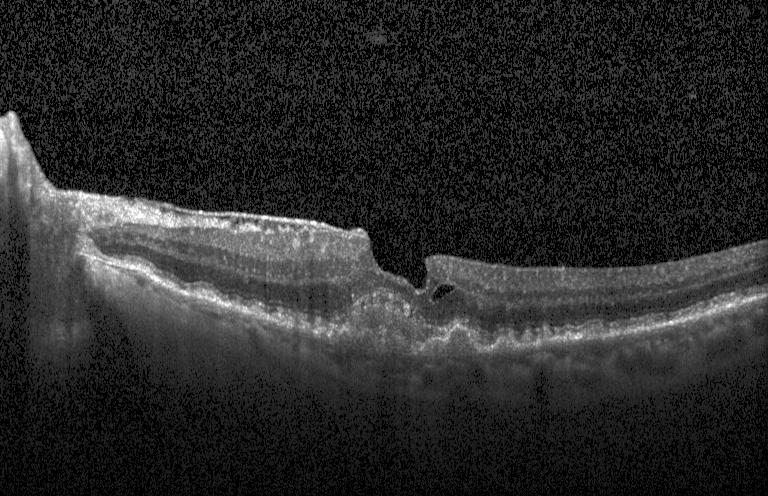 Dx: a choroidal neovascular membrane.